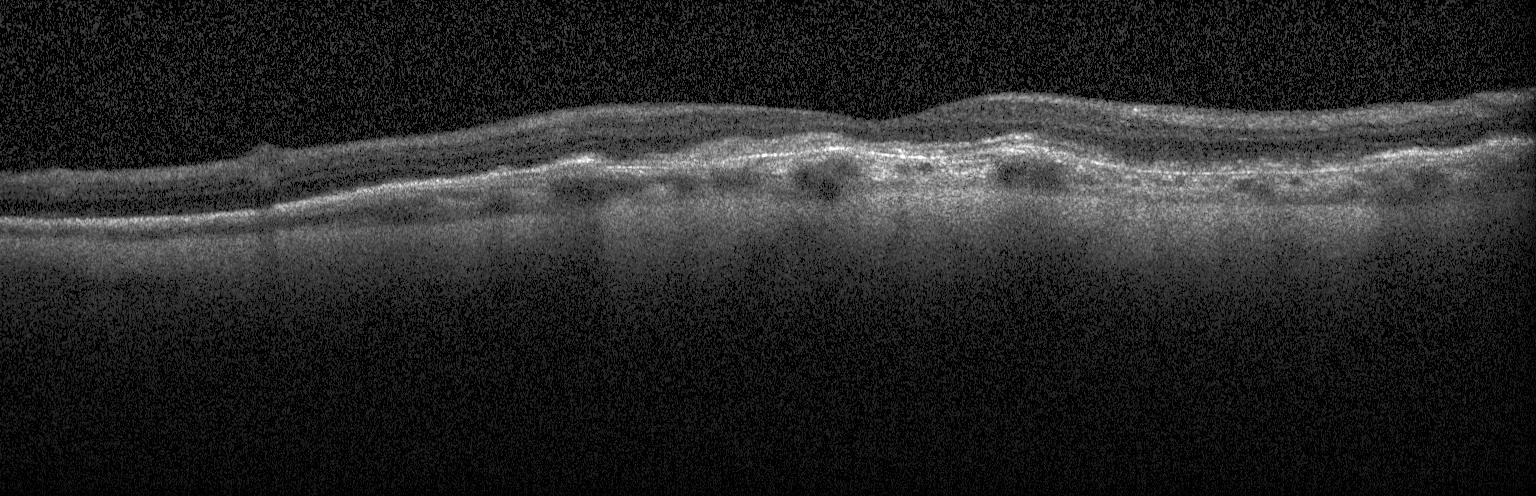 Finding: a choroidal neovascular membrane.